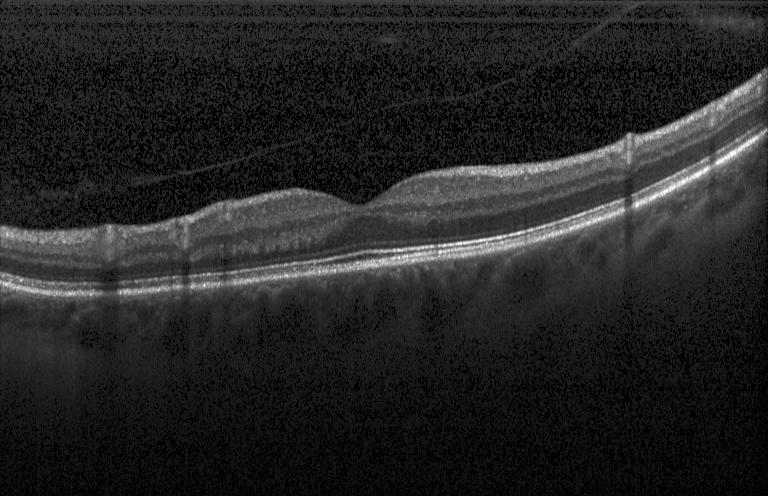 Finding: neither CNV, DME, nor drusen.